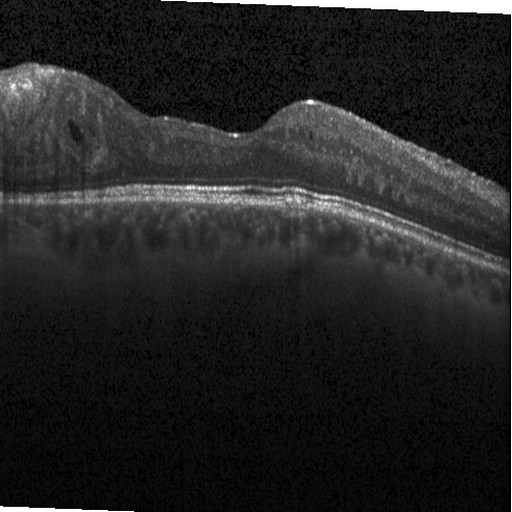
SD-OCT, optical coherence tomography B-scan, centered on the fovea.
Diagnosis: DME.